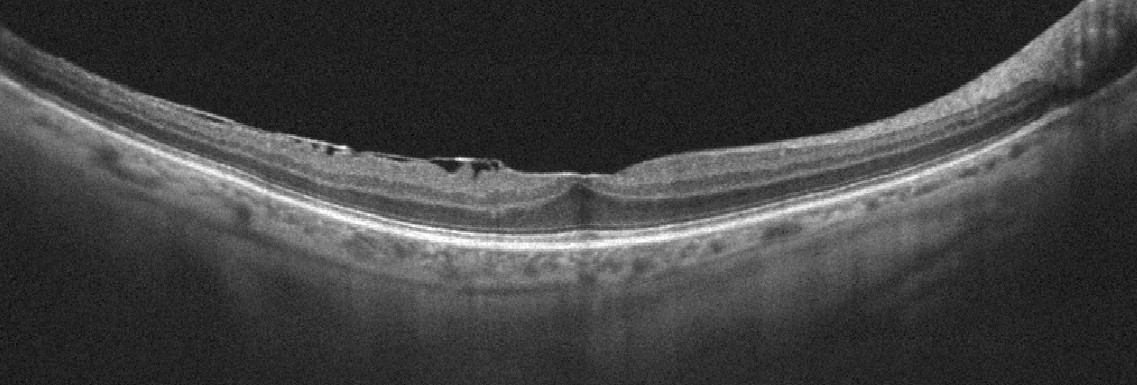

Optical coherence tomography scan — The scan shows epiretinal membrane.